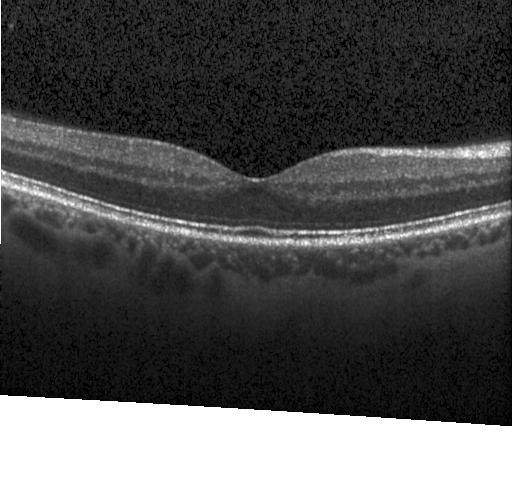 Acquired on a Heidelberg Spectralis, SD-OCT, through the macula, retinal OCT B-scan. Assessment: no CNV, DME, or drusen.